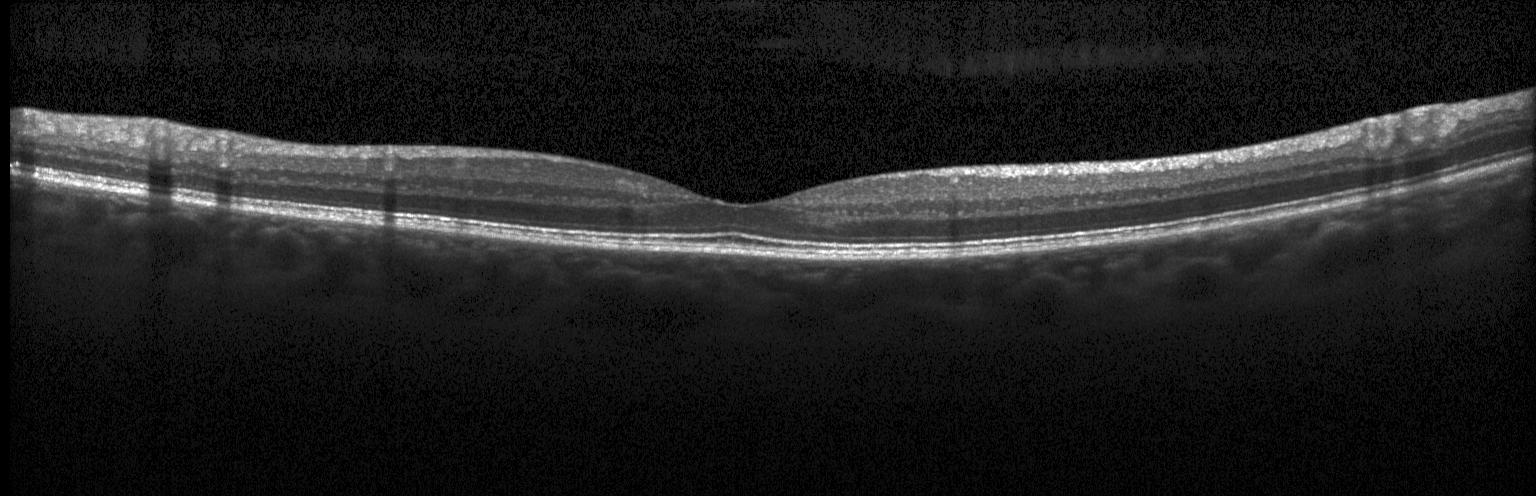 SD-OCT · OCT line scan
Macular OCT: no evidence of choroidal neovascularization, diabetic macular edema, or drusen.